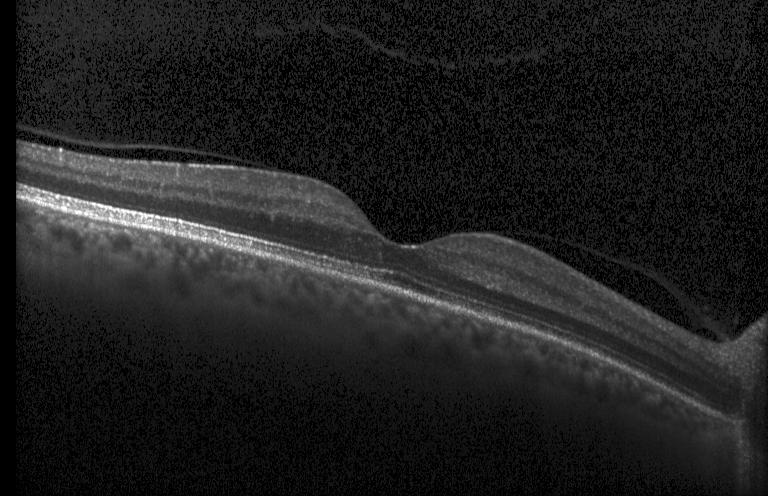 Spectral-domain optical coherence tomography; OCT B-scan; instrument: Heidelberg Spectralis.
OCT finding: no choroidal neovascularization, diabetic macular edema, or drusen.